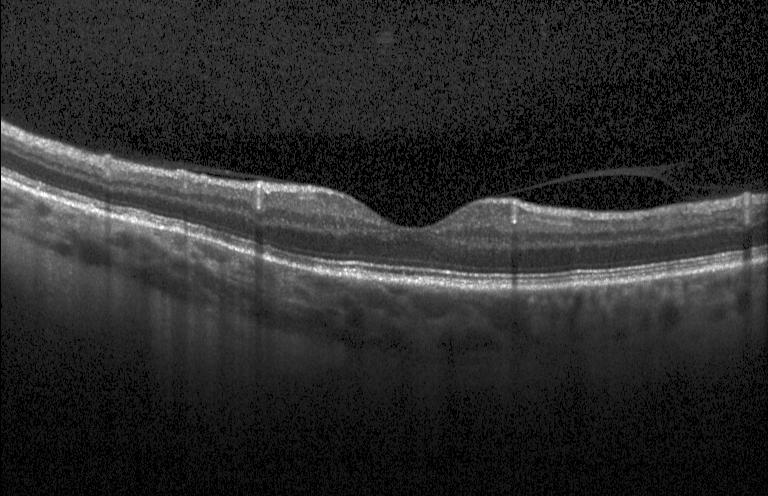

Diagnosis: no choroidal neovascularization, diabetic macular edema, or drusen.